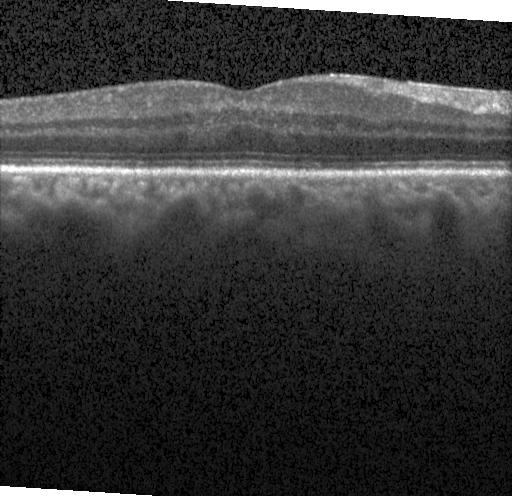
Finding: no choroidal neovascularization, no diabetic macular edema, and no drusen.